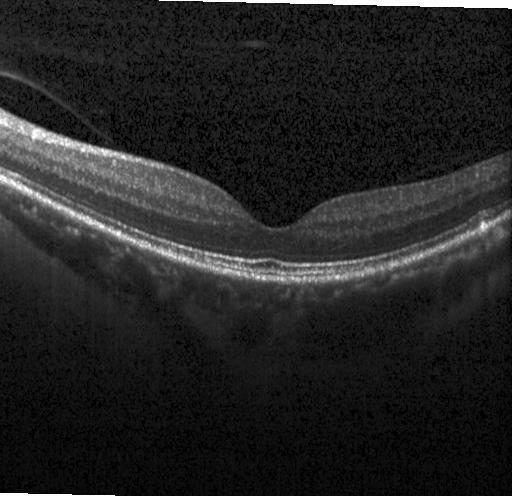

Retinal OCT cross-section. Spectral-domain optical coherence tomography. Acquired on a Heidelberg Spectralis — Impression: no choroidal neovascularization, no diabetic macular edema, and no drusen.